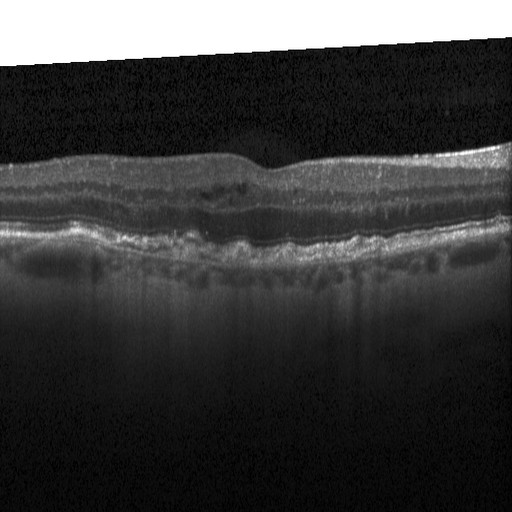

Through the macula, retinal OCT B-scan, spectral-domain OCT, instrument: Heidelberg Spectralis. Diagnosis: DME.